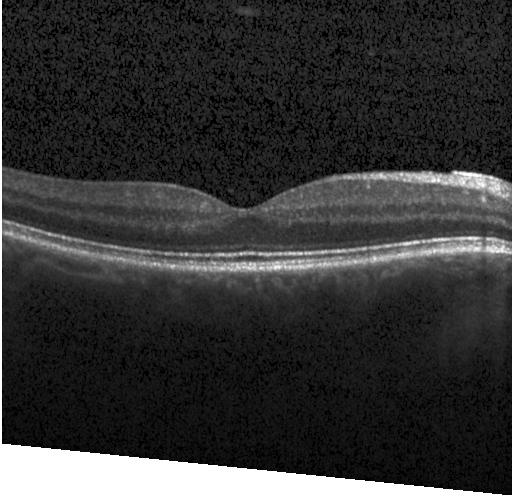 Impression: no choroidal neovascularization, no diabetic macular edema, and no drusen.